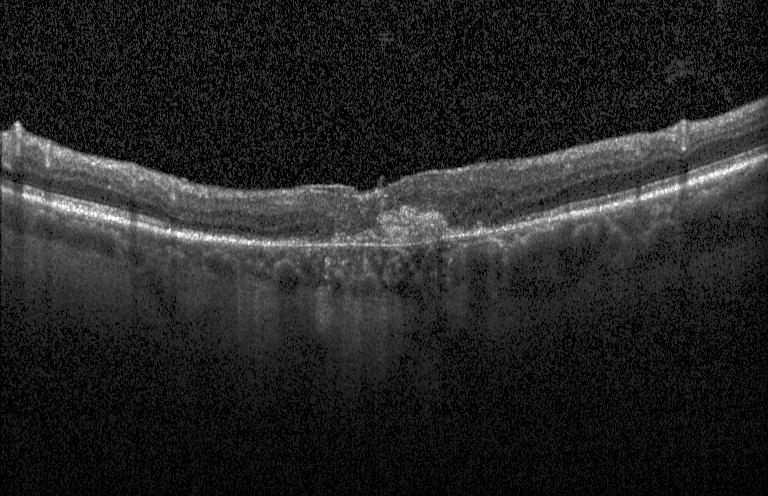
Spectral-domain optical coherence tomography, Heidelberg Spectralis, optical coherence tomography scan — Dx: a choroidal neovascular membrane.